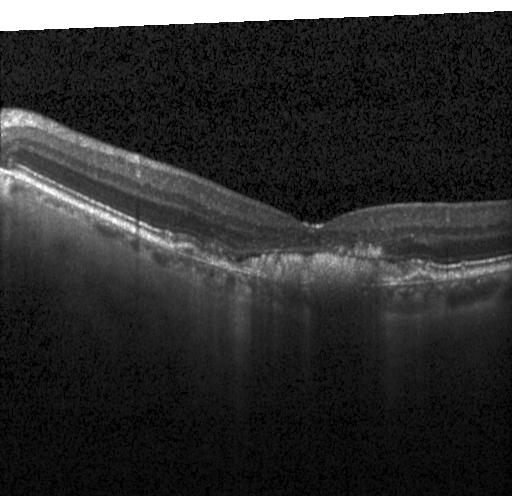

Through the macula, SD-OCT, retinal OCT cross-section. The scan shows choroidal neovascularization (CNV).